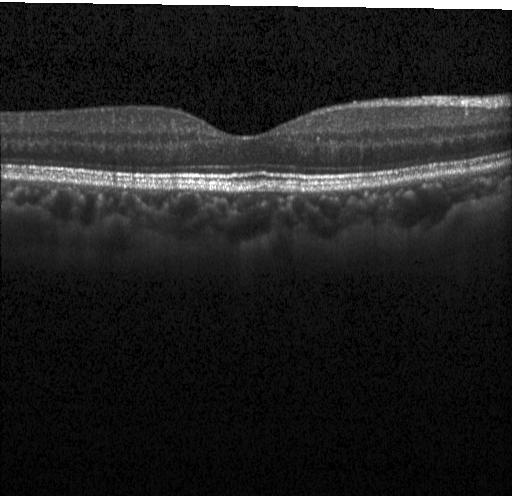

Finding: no CNV, DME, or drusen.